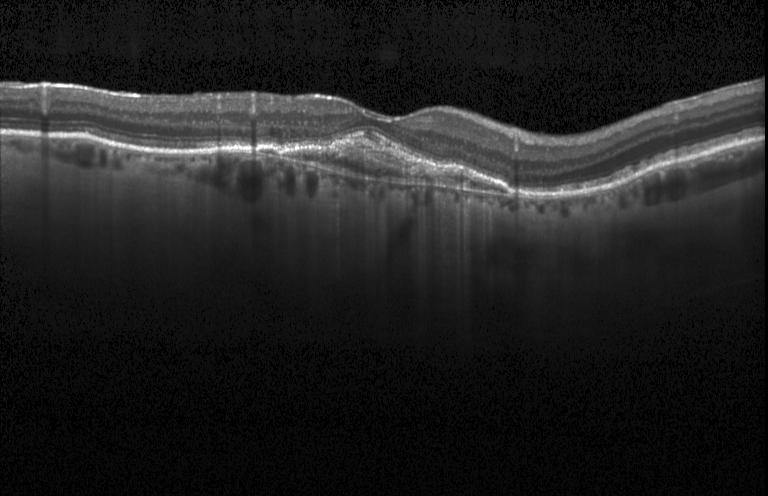

Optical coherence tomography B-scan. Heidelberg Spectralis. Spectral-domain OCT. Horizontal scan through the fovea.
This B-scan demonstrates choroidal neovascularization (CNV).